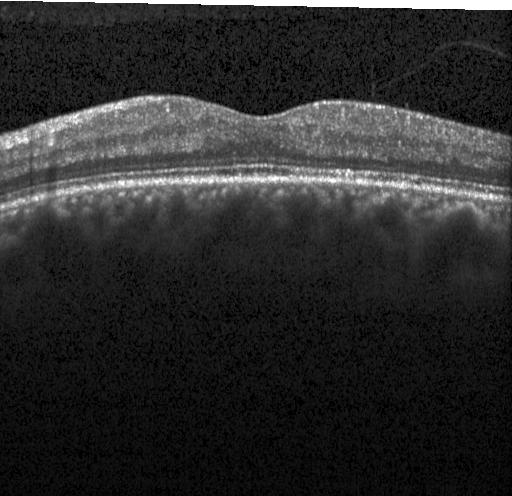 Spectral-domain optical coherence tomography. Retinal OCT B-scan. Heidelberg Spectralis. Diagnosis: no choroidal neovascularization, no diabetic macular edema, and no drusen.